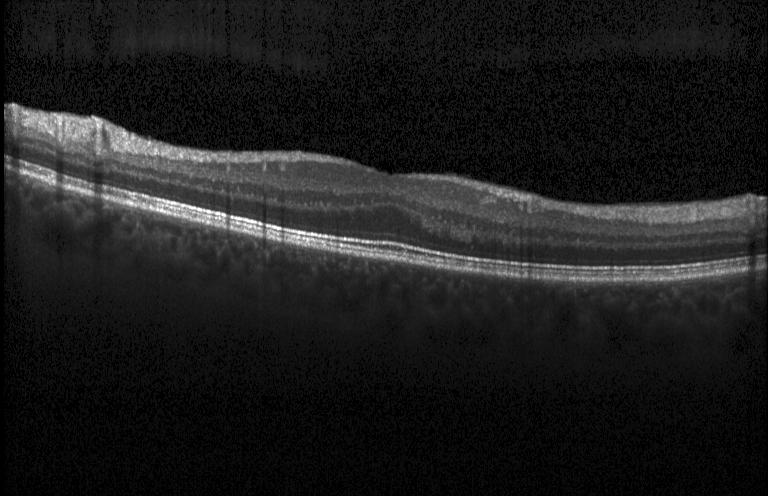 Optical coherence tomography B-scan; fovea-centered
Assessment: no evidence of choroidal neovascularization, diabetic macular edema, or drusen.